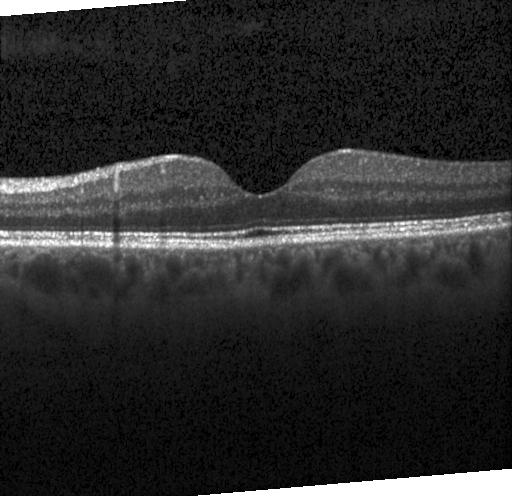
This B-scan demonstrates no choroidal neovascularization, diabetic macular edema, or drusen.